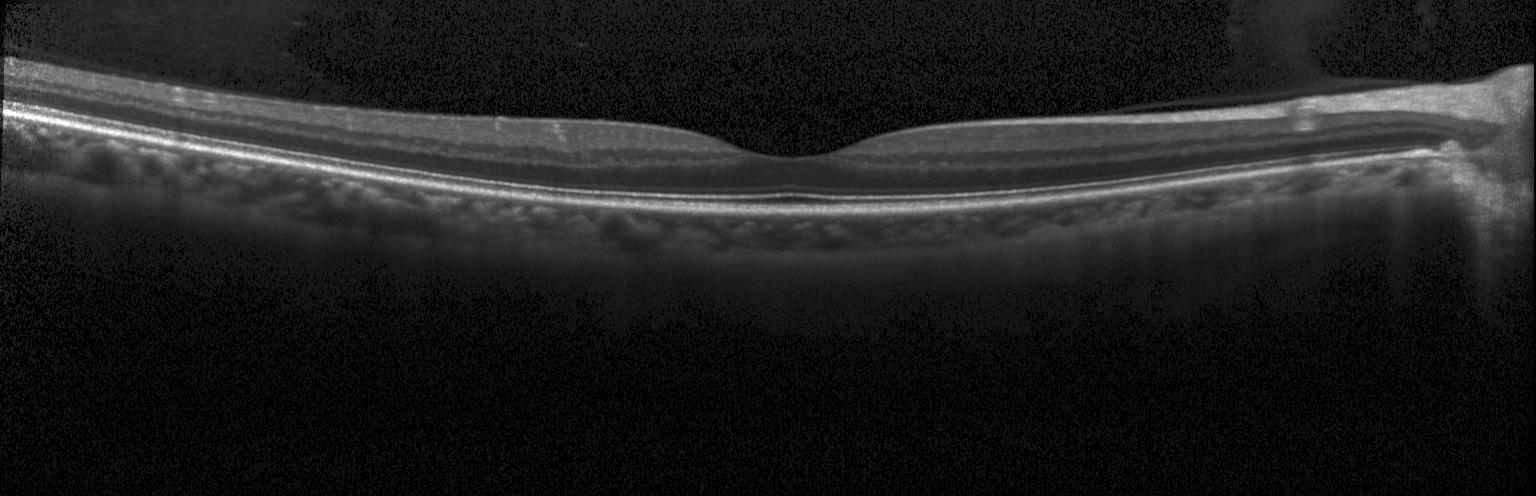

The scan shows no CNV, no DME, and no drusen.